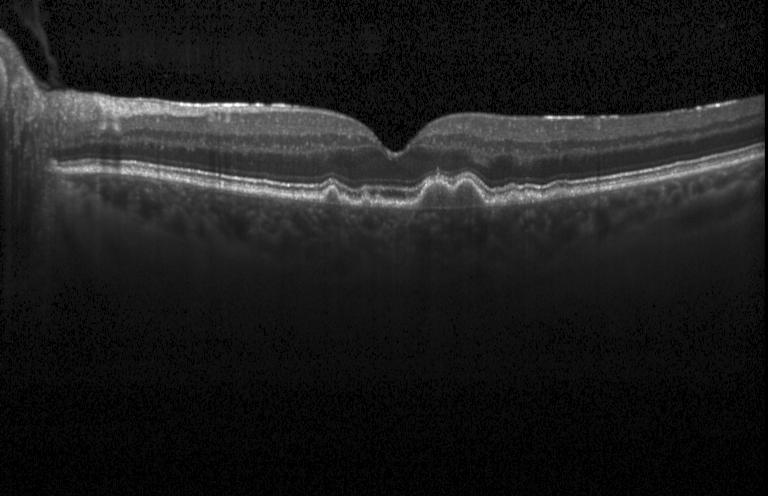 Optical coherence tomography scan. Horizontal scan through the fovea. Instrument: Heidelberg Spectralis
Diagnosis: drusen.